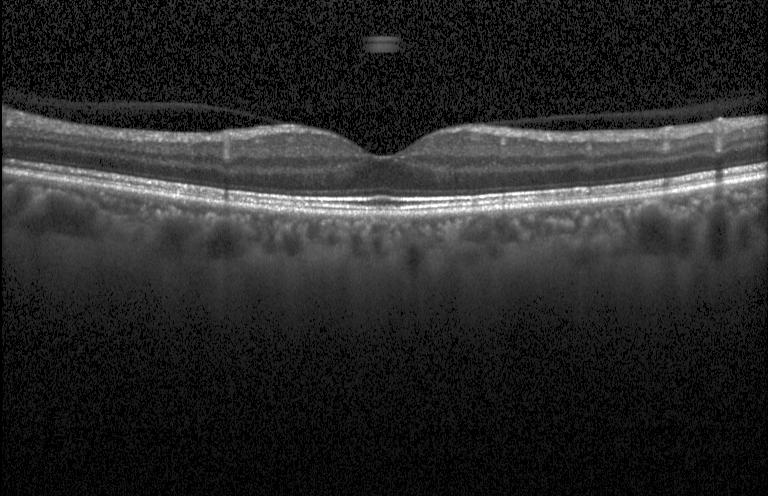
Optical coherence tomography scan · instrument: Heidelberg Spectralis
Finding: no evidence of CNV, DME, or drusen.